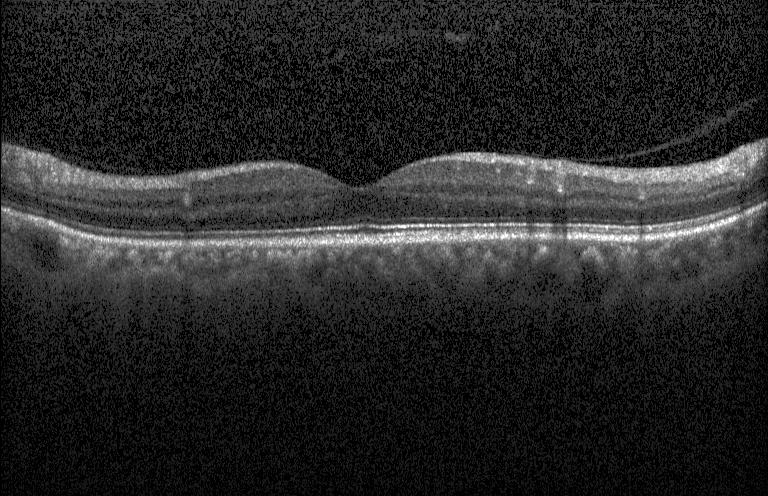 SD-OCT, optical coherence tomography B-scan — Dx: no choroidal neovascularization, diabetic macular edema, or drusen.